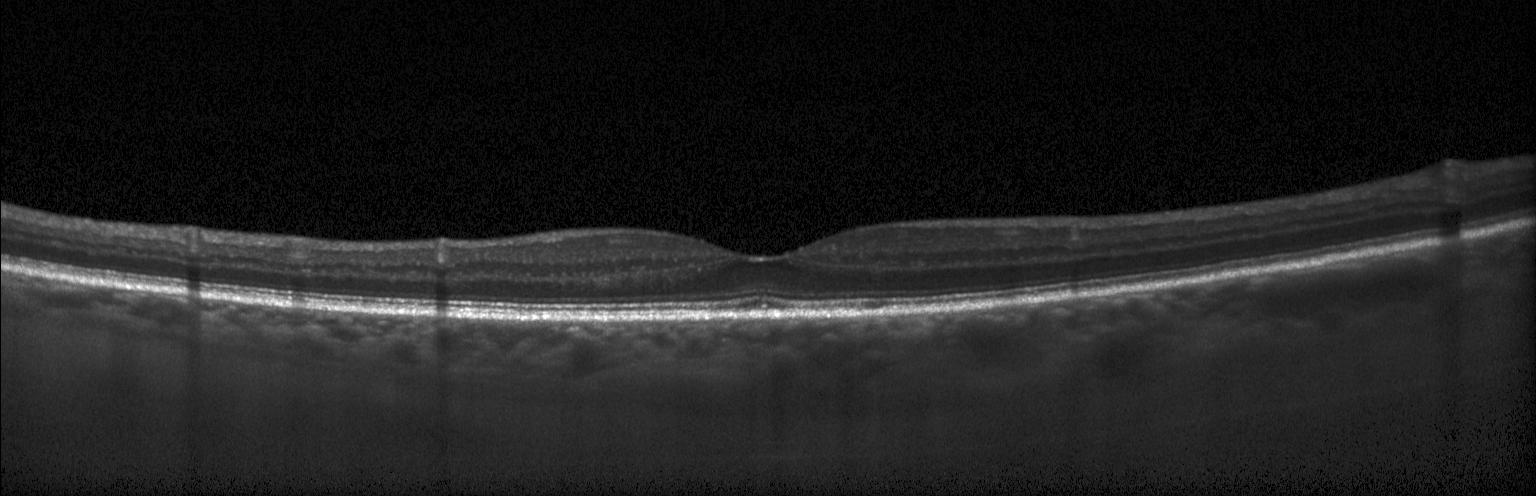 Heidelberg Spectralis; OCT line scan
Finding: no choroidal neovascularization, no diabetic macular edema, and no drusen.